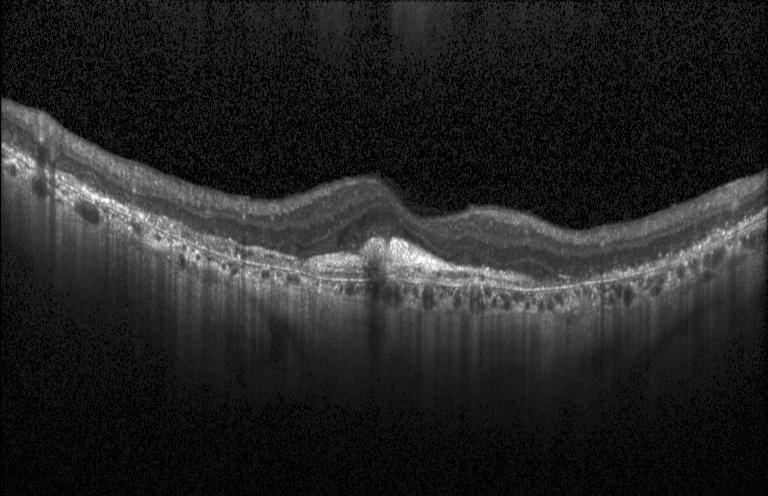 Impression: choroidal neovascularization.